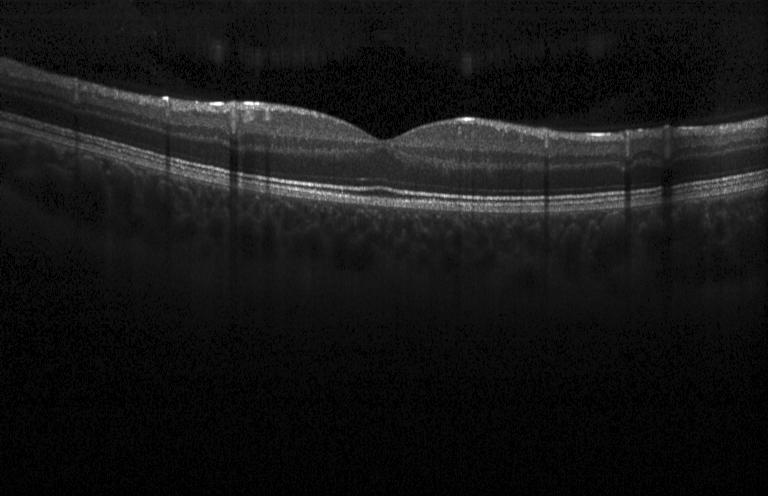 The scan shows no choroidal neovascularization, no diabetic macular edema, and no drusen.